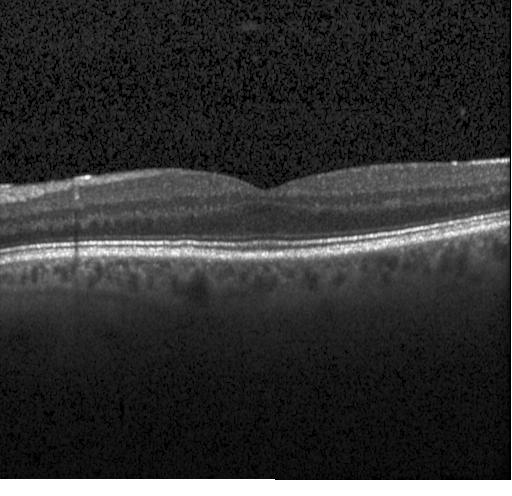

Macular scan; OCT line scan; SD-OCT; Heidelberg Spectralis.
No evidence of choroidal neovascularization, diabetic macular edema, or drusen.